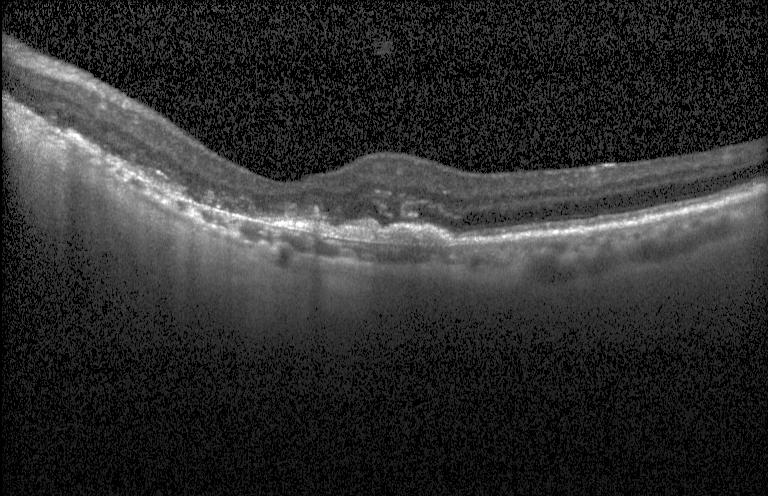 OCT B-scan.
Diagnosis: CNV.